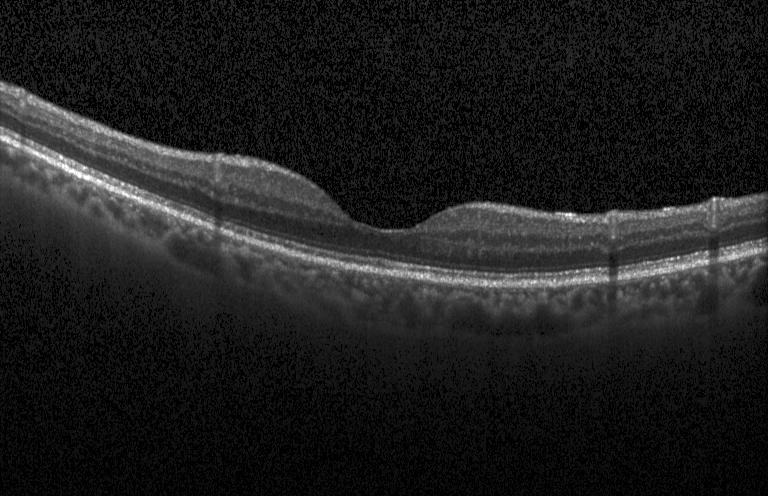

SD-OCT · centered on the fovea · OCT B-scan — Diagnosis: no choroidal neovascularization, no diabetic macular edema, and no drusen.